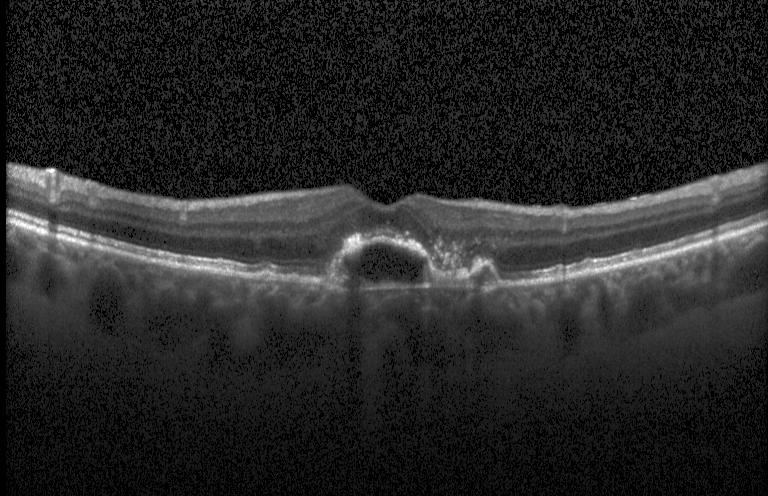

SD-OCT, Heidelberg Spectralis OCT system, macular scan, OCT line scan
Diagnosis: choroidal neovascularization (CNV).